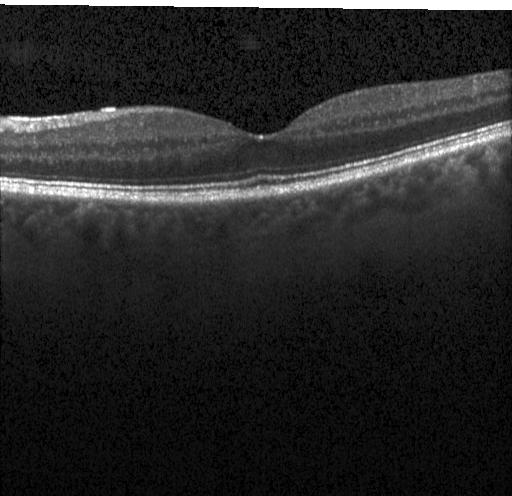

Impression: no evidence of choroidal neovascularization, diabetic macular edema, or drusen.